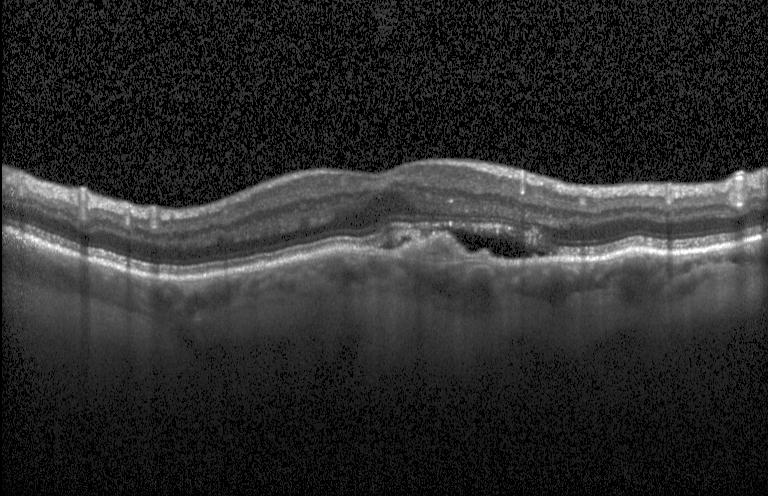 Retinal OCT B-scan.
Diagnosis: a choroidal neovascular membrane.